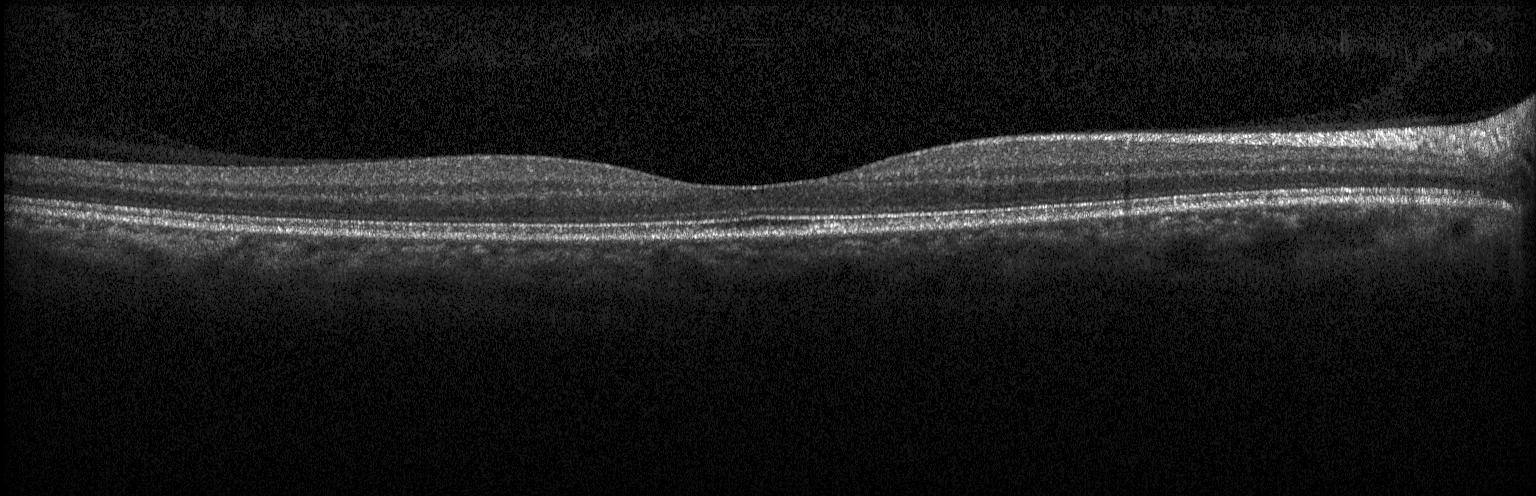
Through the macula, Heidelberg Spectralis, OCT B-scan, spectral-domain optical coherence tomography
No evidence of choroidal neovascularization, diabetic macular edema, or drusen.